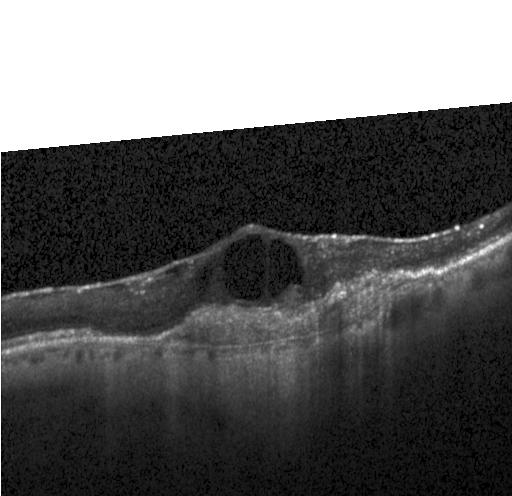 Heidelberg Spectralis OCT system, retinal OCT cross-section — Diagnosis: a choroidal neovascular membrane.